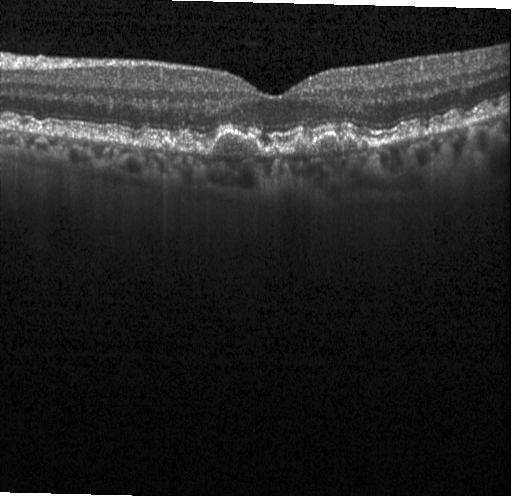 Dx: sub-RPE drusenoid deposits.